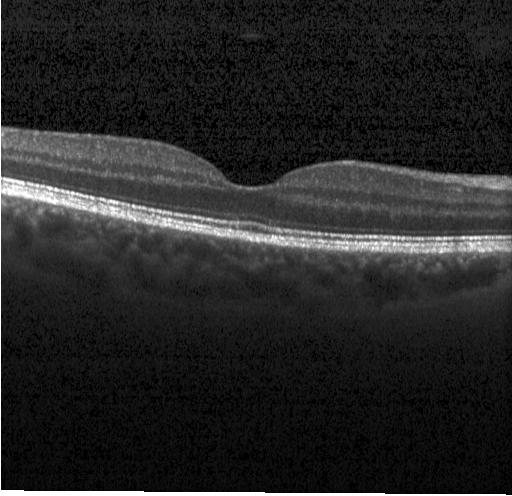 OCT B-scan showing neither choroidal neovascularization, diabetic macular edema, nor drusen.